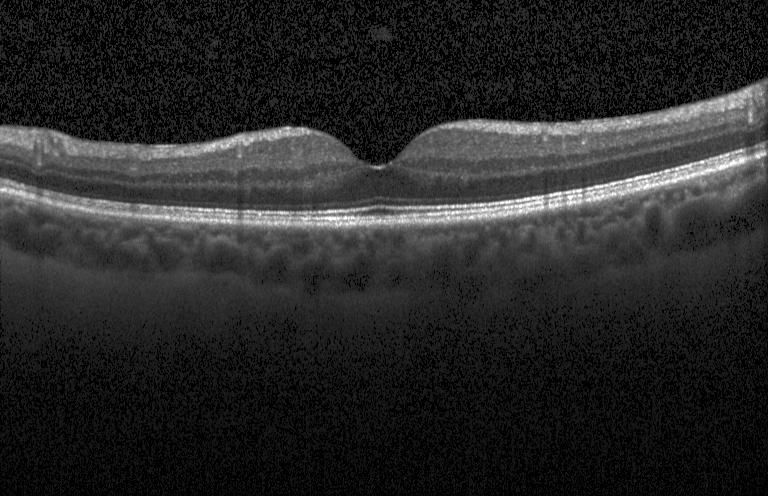

Diagnosis: no choroidal neovascularization, no diabetic macular edema, and no drusen.